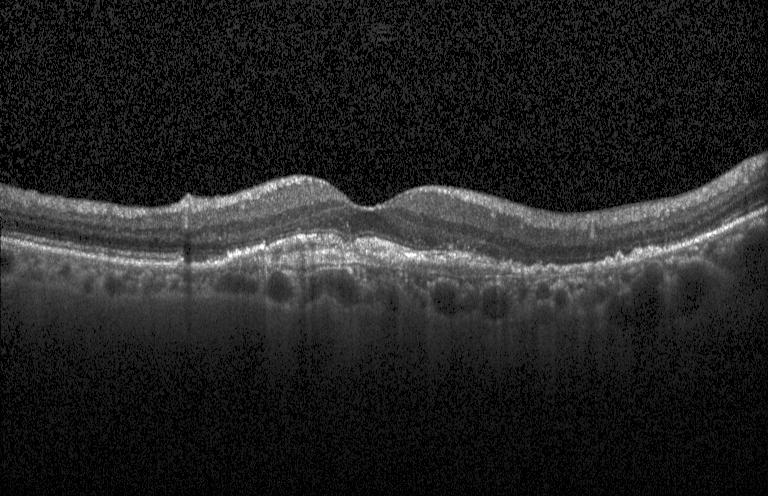

Finding: a choroidal neovascular membrane.